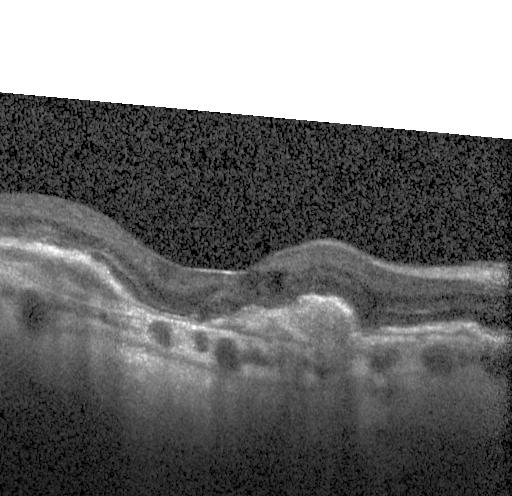
Retinal OCT cross-section
Impression: a choroidal neovascular membrane.